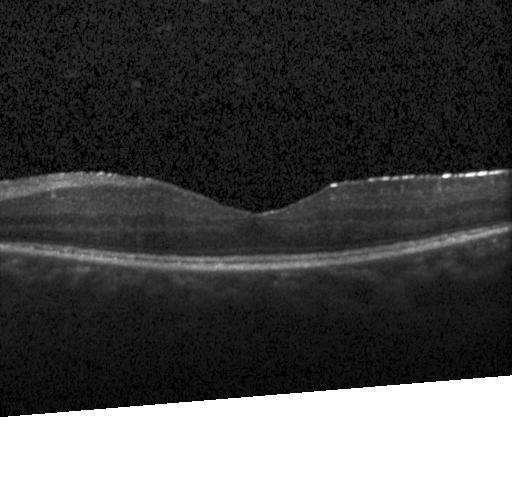 OCT B-scan, macular scan, spectral-domain OCT.
Diagnosis: no evidence of choroidal neovascularization, diabetic macular edema, or drusen.